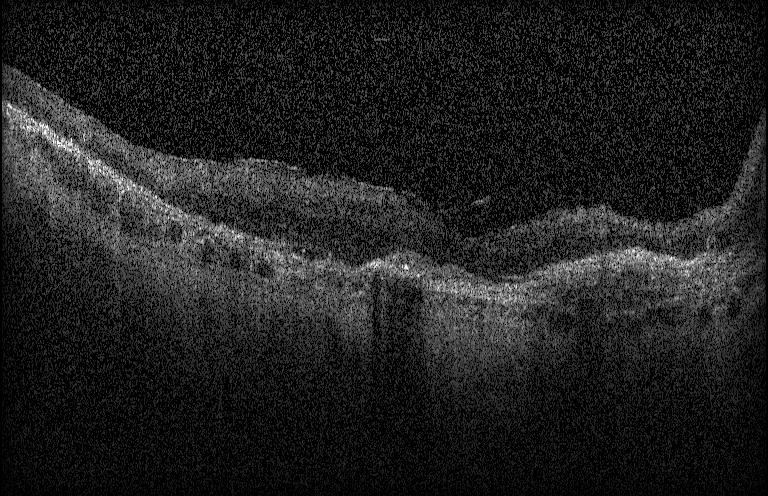

Heidelberg Spectralis OCT system. Macular scan. Retinal OCT cross-section
Assessment: choroidal neovascularization.